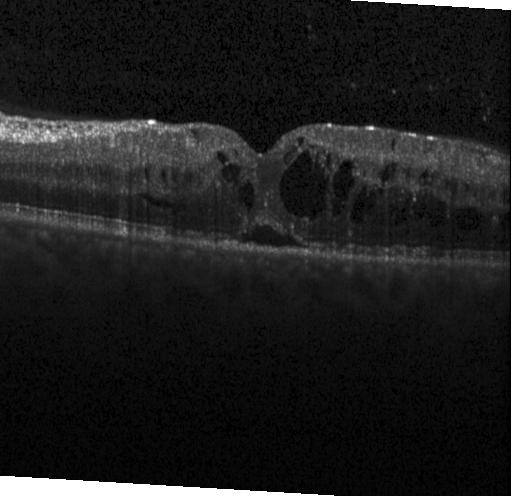
OCT B-scan · horizontal scan through the fovea · instrument: Heidelberg Spectralis · spectral-domain OCT.
Finding: DME.